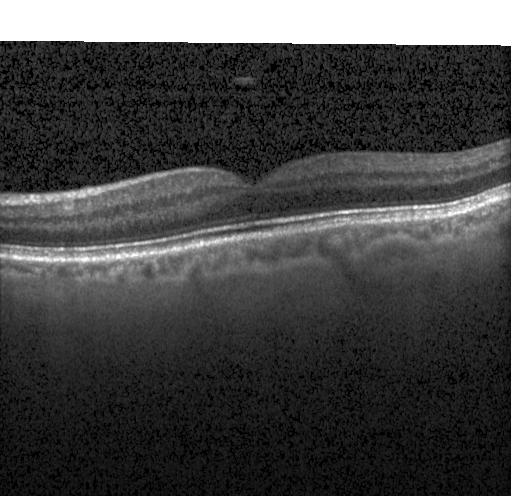 Spectral-domain OCT · OCT line scan · Heidelberg Spectralis. The scan shows no evidence of CNV, DME, or drusen.